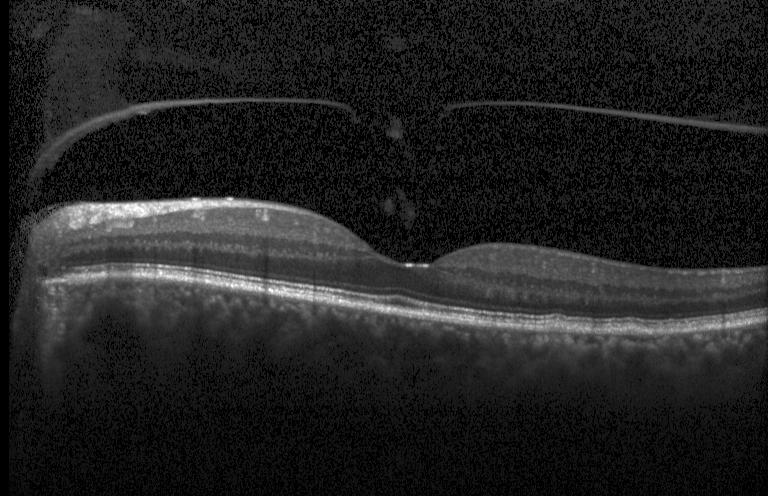

Retinal OCT cross-section; macular scan. Finding: no CNV, DME, or drusen.